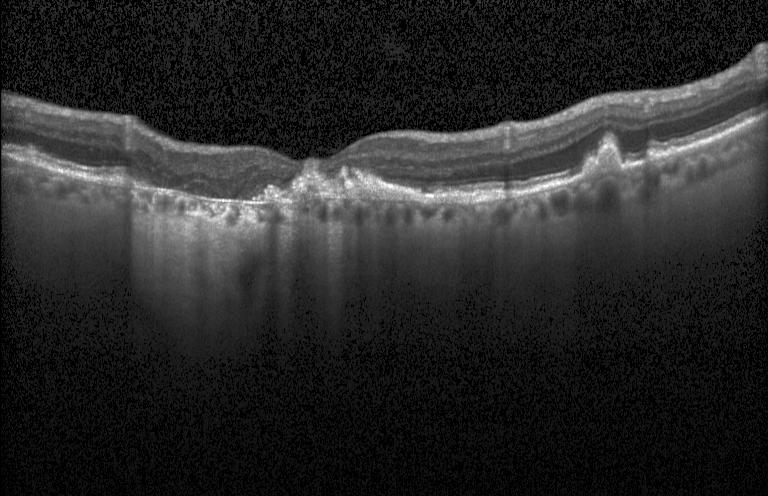

Macular OCT: CNV.